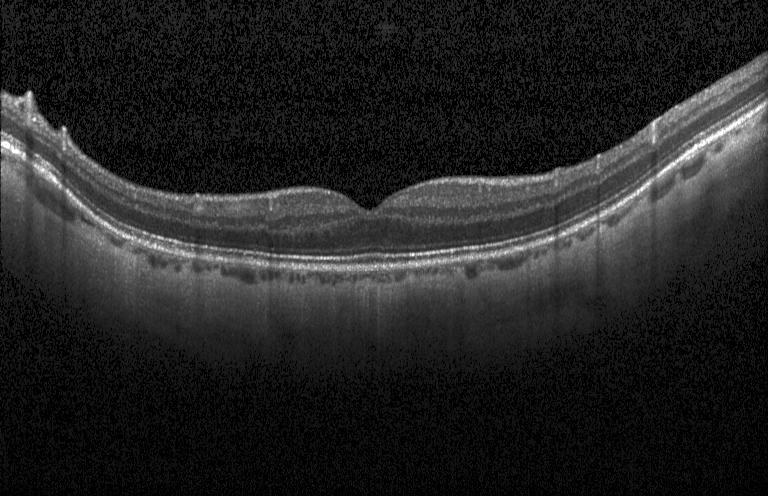 OCT B-scan.
Finding: no CNV, no DME, and no drusen.